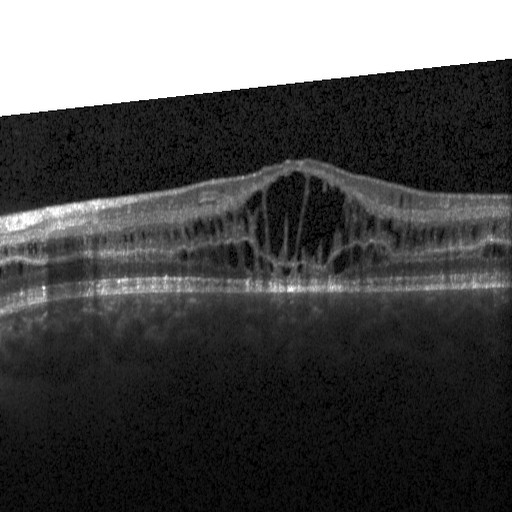

Retinal OCT cross-section showing diabetic macular edema.